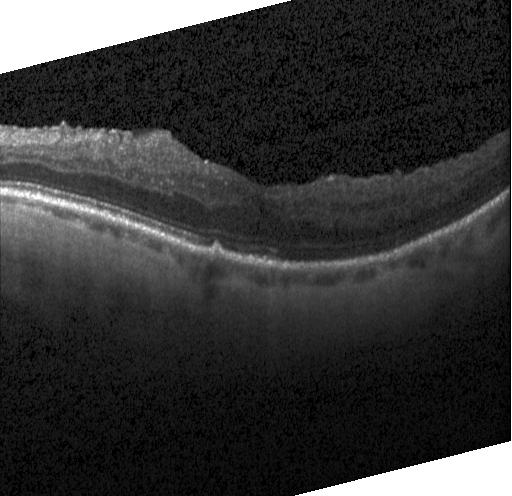
Acquired on a Heidelberg Spectralis · OCT B-scan. Assessment: multiple drusen.